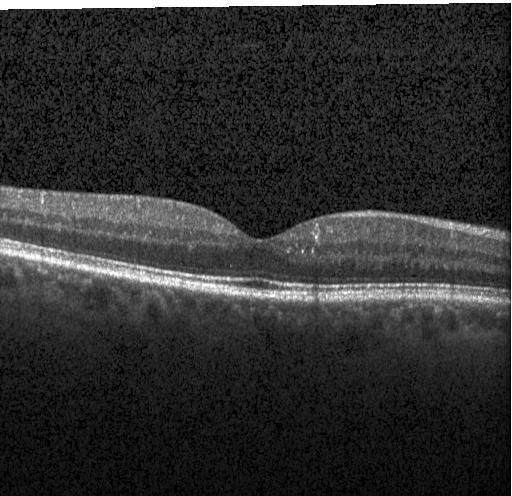

Retinal OCT cross-section
Finding: no choroidal neovascularization, diabetic macular edema, or drusen.